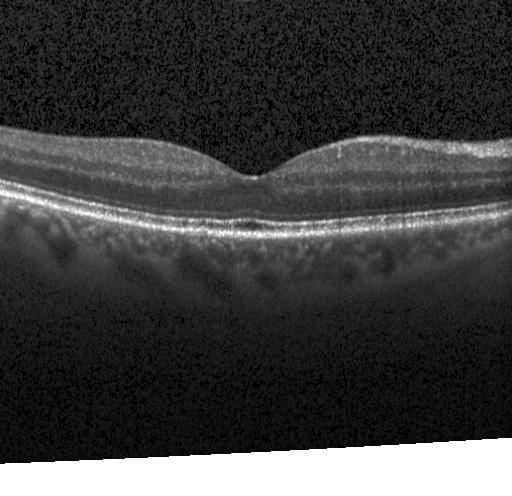

Retinal OCT B-scan · acquired on a Heidelberg Spectralis. Macular OCT: neither choroidal neovascularization, diabetic macular edema, nor drusen.